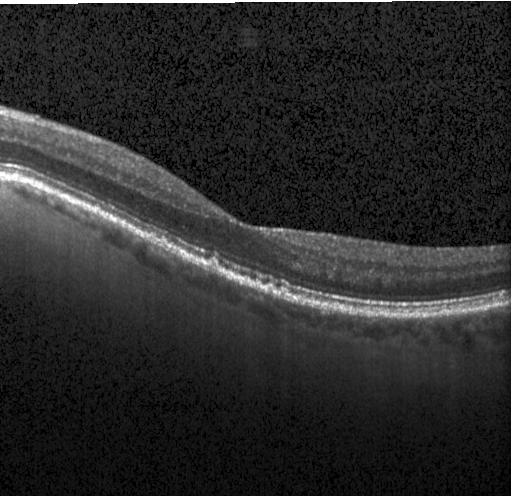
OCT line scan — Assessment: multiple drusen.